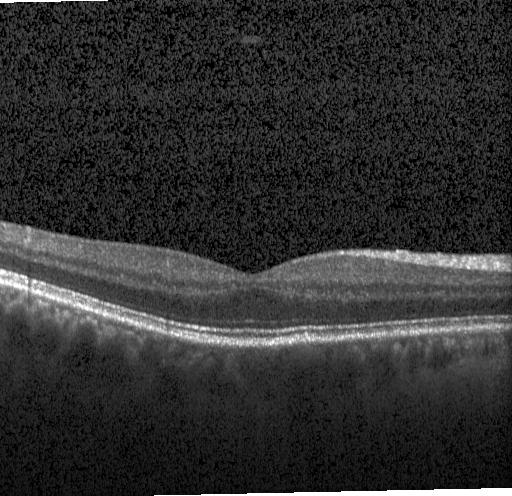 Heidelberg Spectralis OCT system. OCT B-scan. The scan shows no evidence of choroidal neovascularization, diabetic macular edema, or drusen.